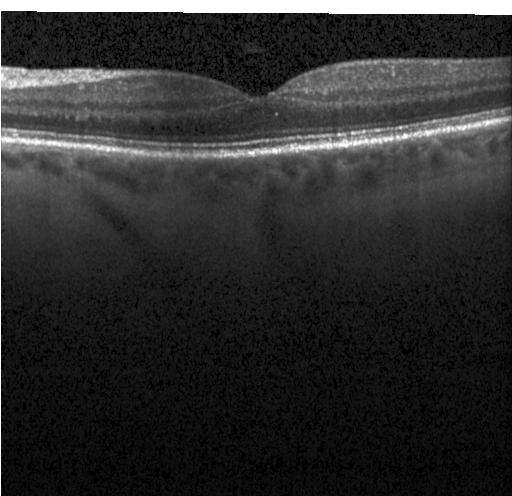 OCT line scan.
Dx: no choroidal neovascularization, diabetic macular edema, or drusen.